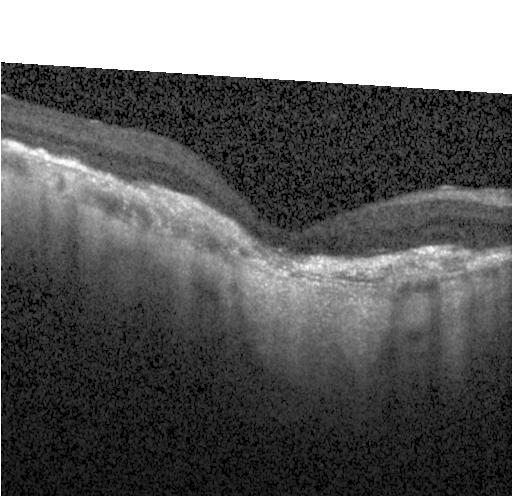 Diagnosis: choroidal neovascularization.